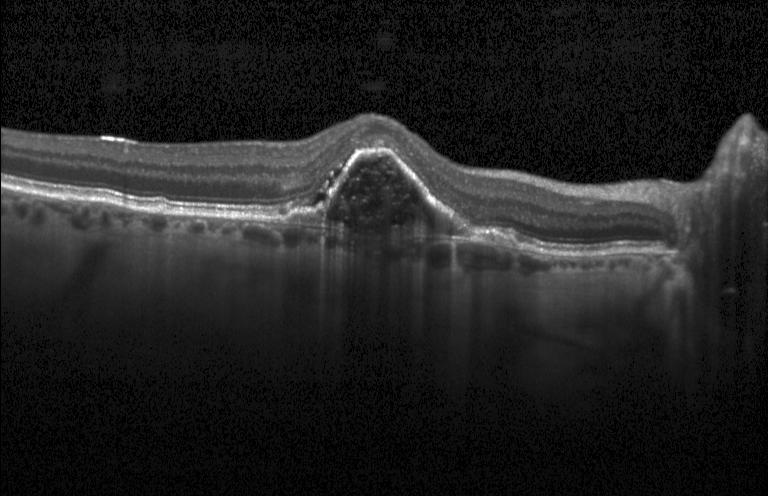

Instrument: Heidelberg Spectralis, retinal OCT cross-section.
Finding: choroidal neovascularization.